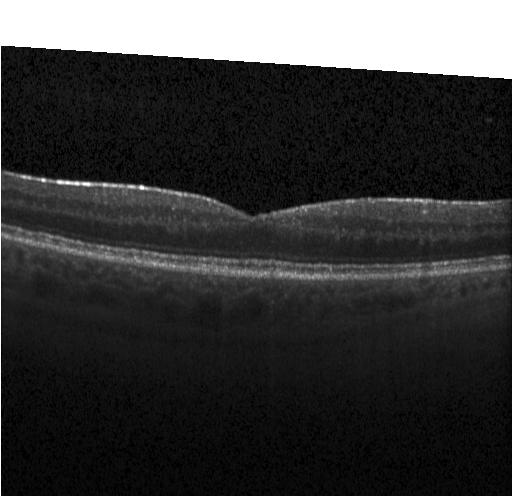 SD-OCT, Heidelberg Spectralis OCT system, OCT line scan — Assessment: neither choroidal neovascularization, diabetic macular edema, nor drusen.